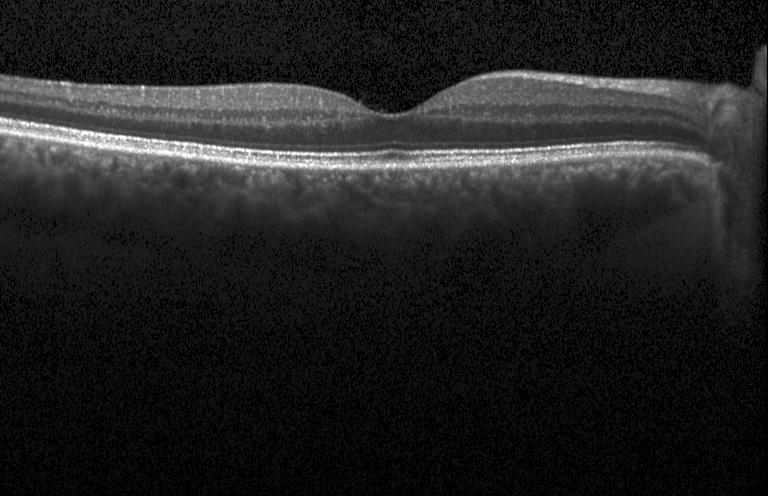 Optical coherence tomography B-scan. Instrument: Heidelberg Spectralis. Dx: no choroidal neovascularization, diabetic macular edema, or drusen.